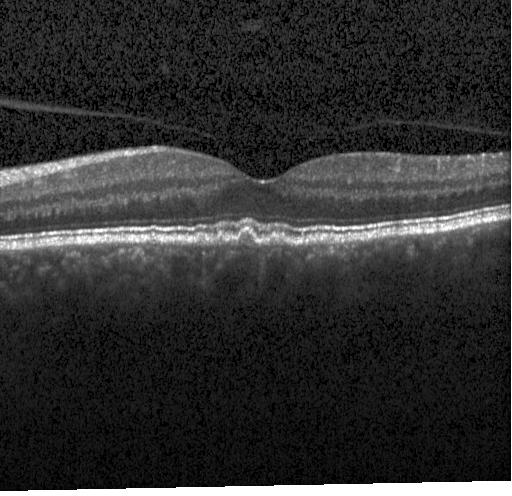

Optical coherence tomography scan. Assessment: multiple drusen.